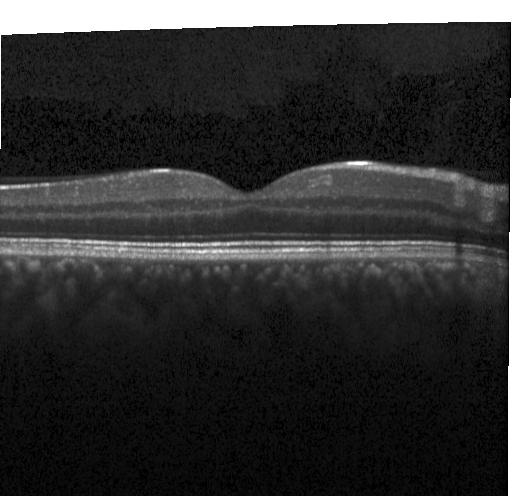 No choroidal neovascularization, no diabetic macular edema, and no drusen.